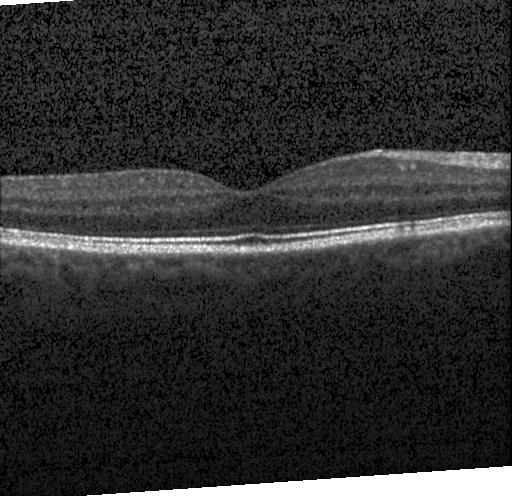

This B-scan demonstrates neither choroidal neovascularization, diabetic macular edema, nor drusen.